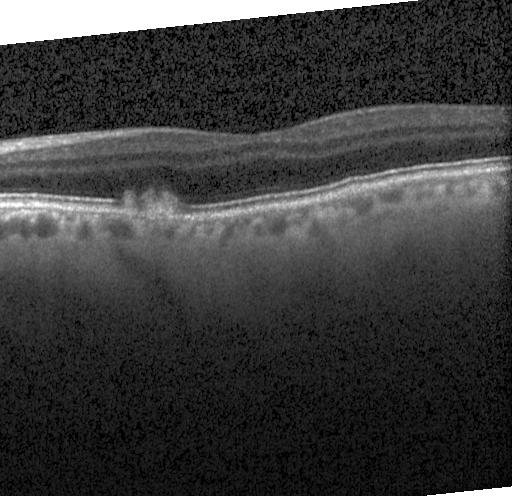

Assessment: CNV.